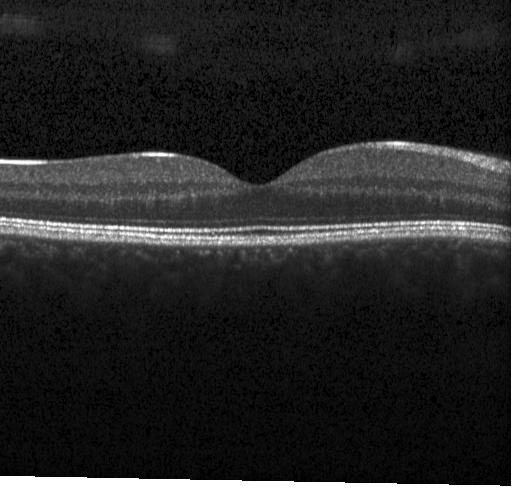 Optical coherence tomography B-scan, through the macula. The scan shows no evidence of choroidal neovascularization, diabetic macular edema, or drusen.